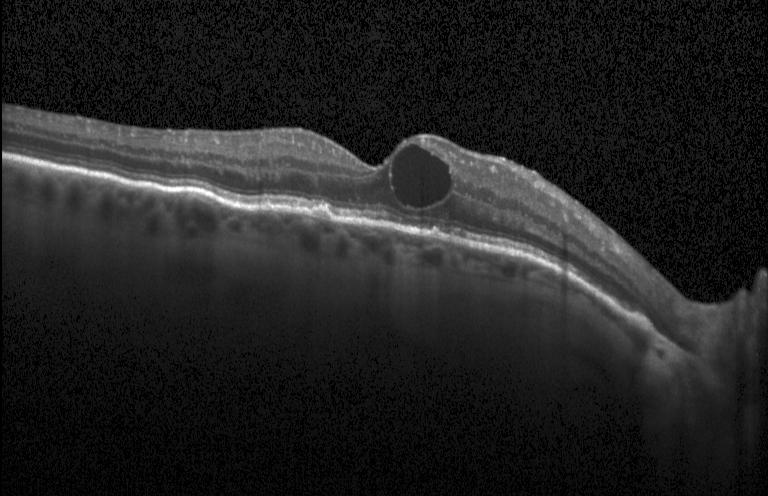
Diagnosis: a choroidal neovascular membrane.